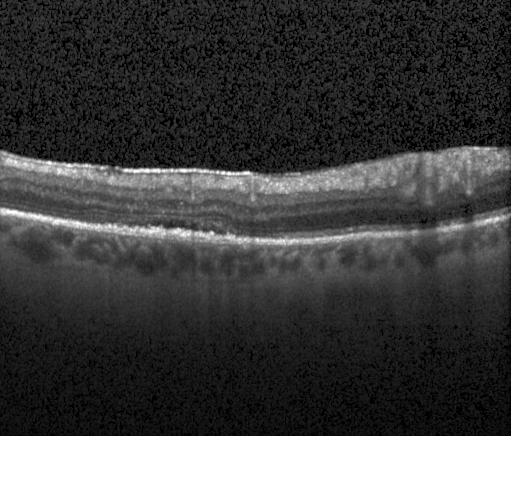 Instrument: Heidelberg Spectralis, OCT line scan. Finding: choroidal neovascularization.